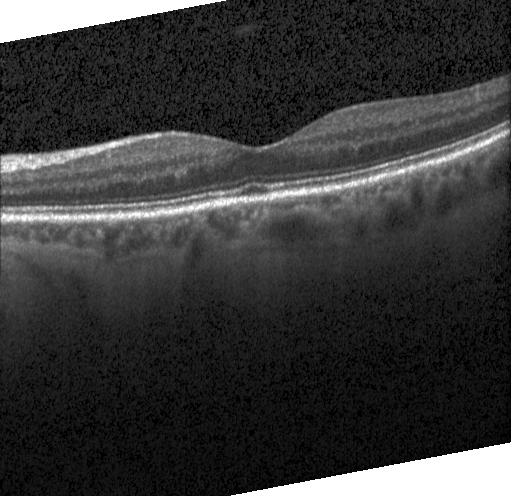
Spectral-domain OCT B-scan: no evidence of CNV, DME, or drusen.